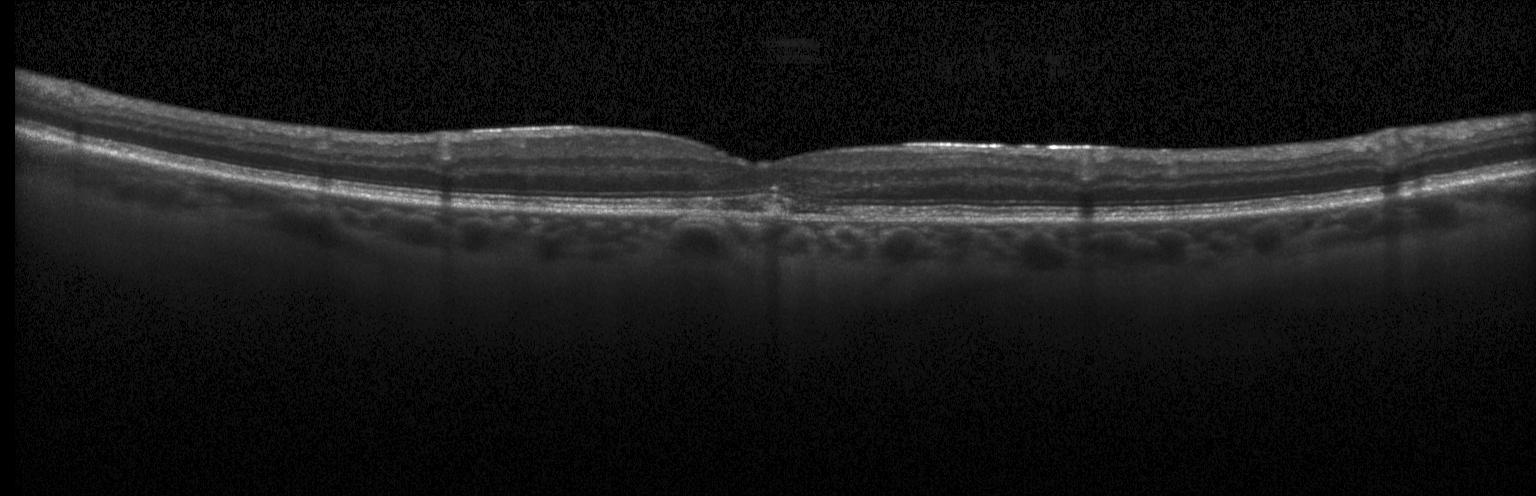
Fovea-centered · instrument: Heidelberg Spectralis · retinal OCT B-scan.
Finding: choroidal neovascularization.